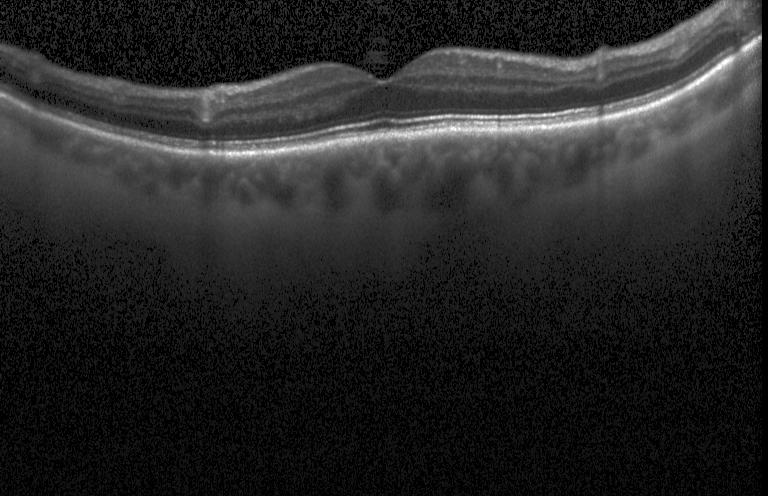

Optical coherence tomography scan. Diagnosis: neither CNV, DME, nor drusen.